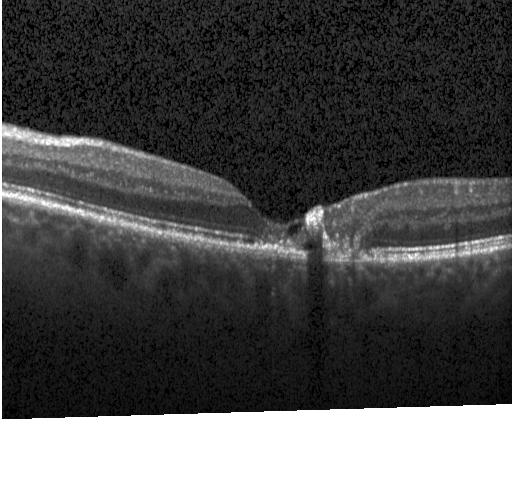 Optical coherence tomography scan.
Impression: choroidal neovascularization (CNV).